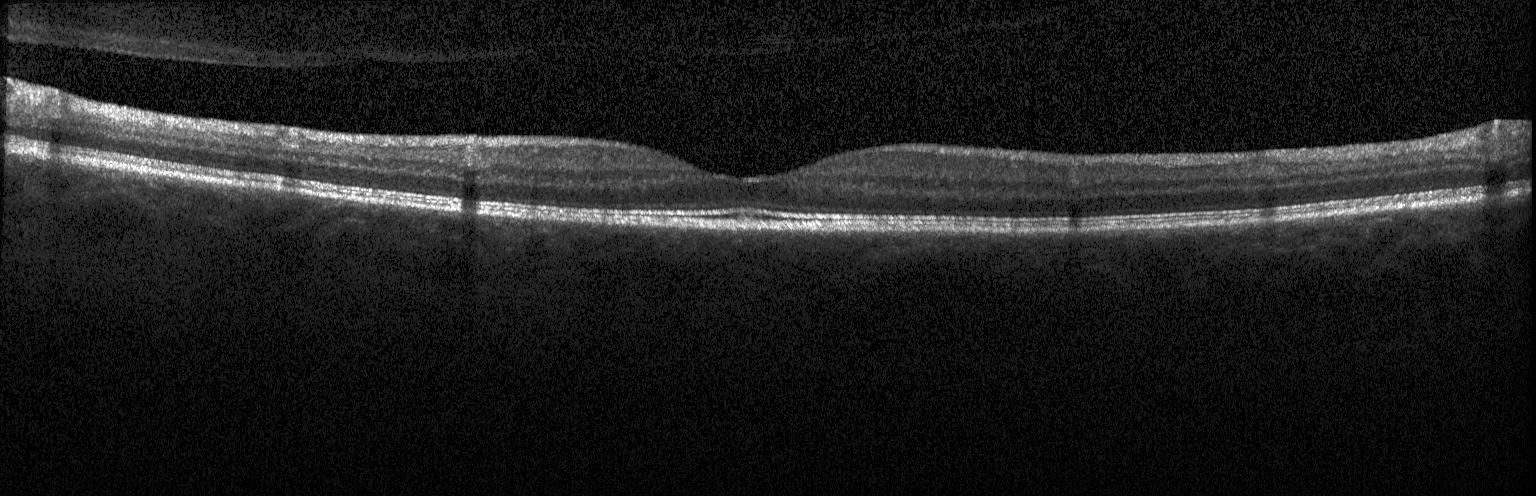
Optical coherence tomography B-scan. OCT finding: no CNV, DME, or drusen.